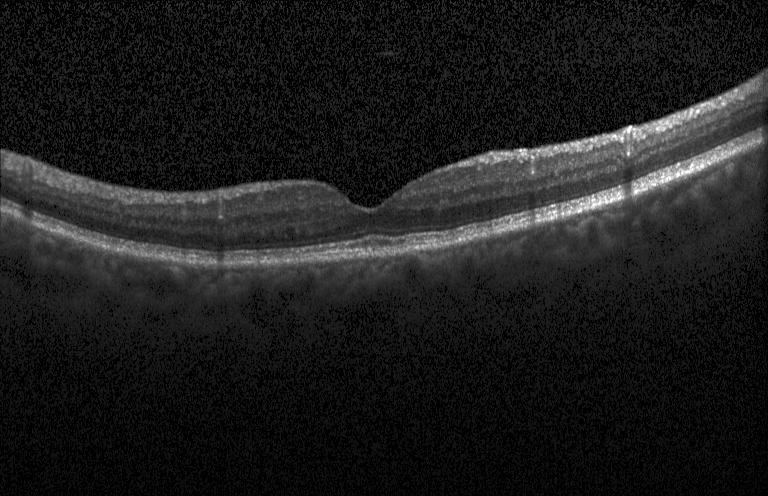
Through the macula, optical coherence tomography B-scan. Diagnosis: neither choroidal neovascularization, diabetic macular edema, nor drusen.